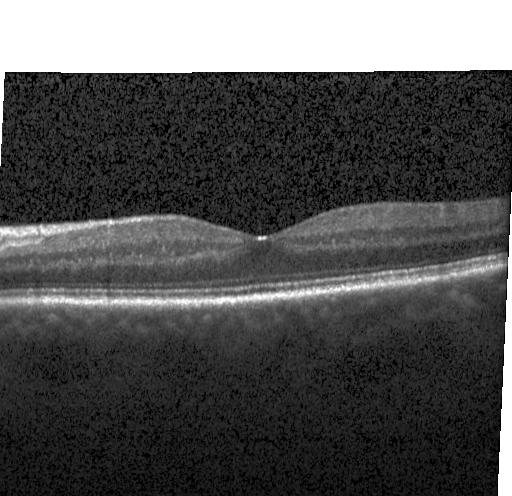 Spectral-domain OCT B-scan: no choroidal neovascularization, diabetic macular edema, or drusen.